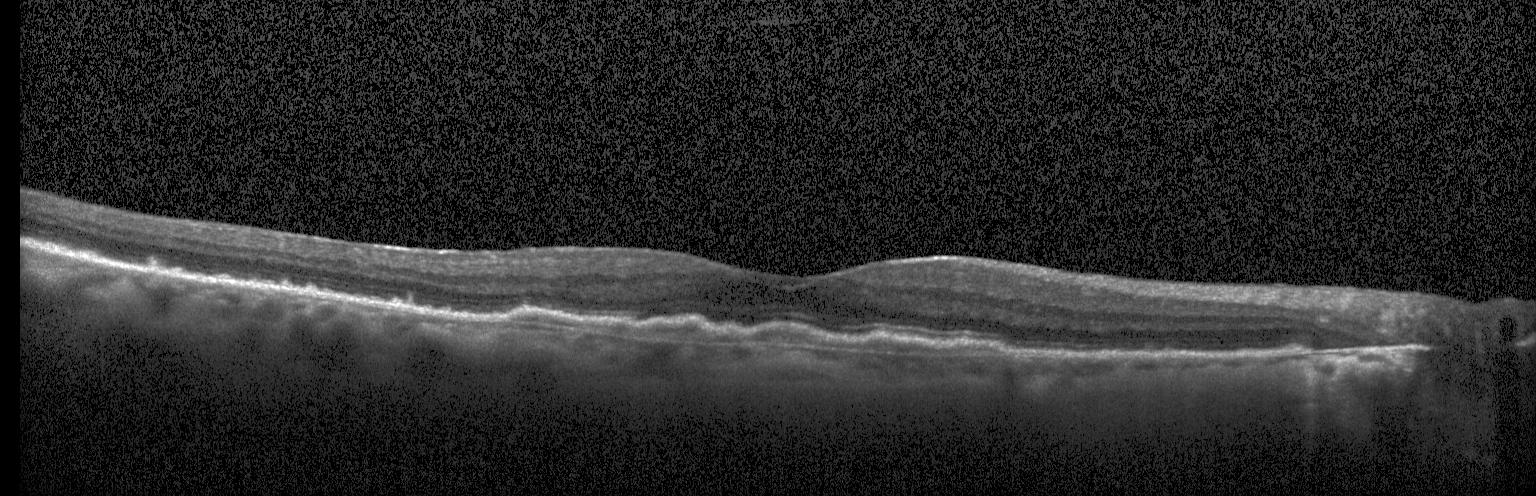

The scan shows a choroidal neovascular membrane.